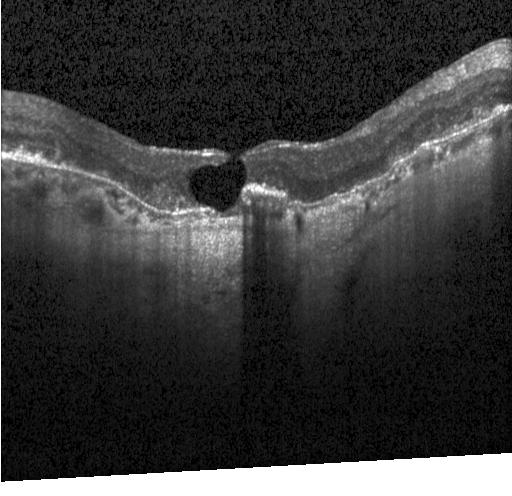

Optical coherence tomography B-scan. SD-OCT. Heidelberg Spectralis
Finding: choroidal neovascularization.